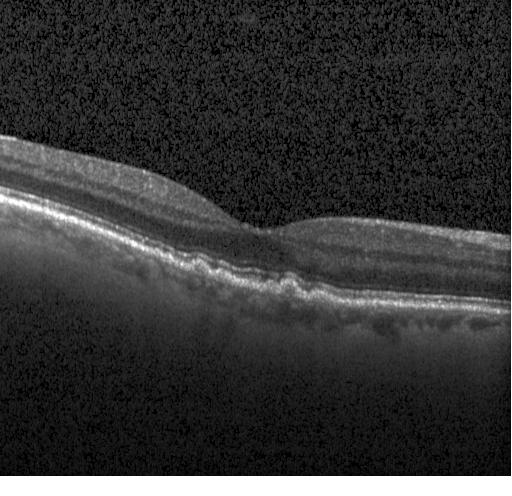 Retinal OCT cross-section showing drusen.